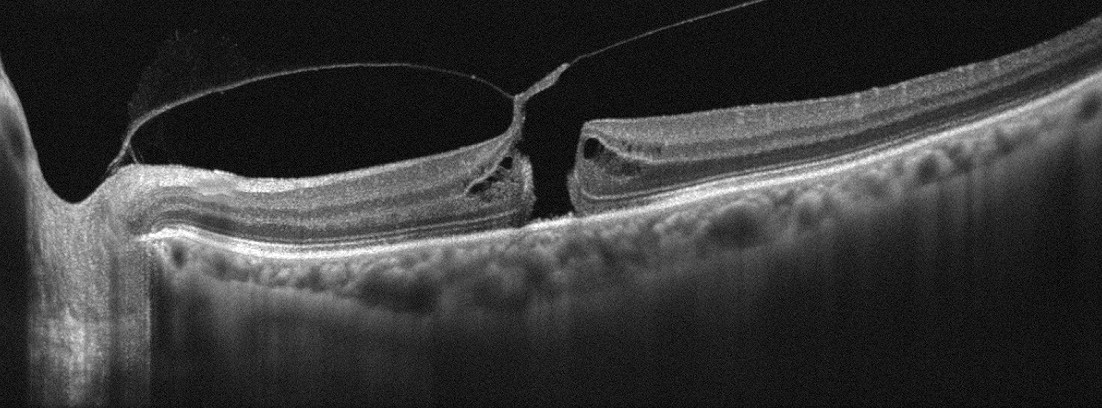
OCT line scan · acquired on an Optovue Avanti RTVue XR. Diagnosis: VID.